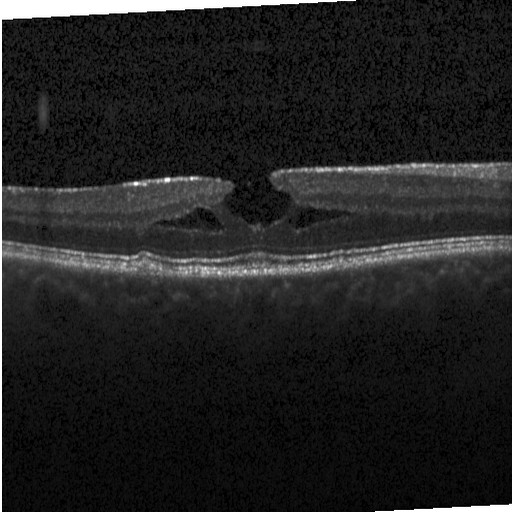

Spectral-domain optical coherence tomography, horizontal scan through the fovea, Heidelberg Spectralis, OCT line scan. Diagnosis: diabetic macular edema (DME).